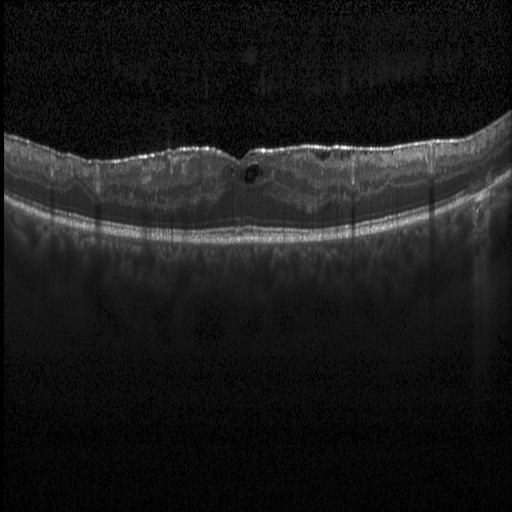
Retinal OCT B-scan; fovea-centered — This B-scan demonstrates diabetic macular edema (DME).